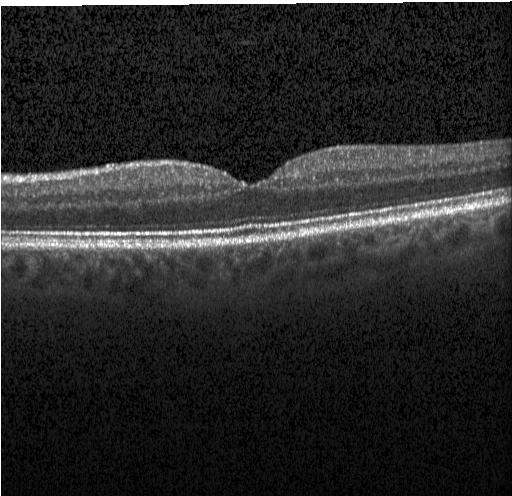 The scan shows neither choroidal neovascularization, diabetic macular edema, nor drusen.